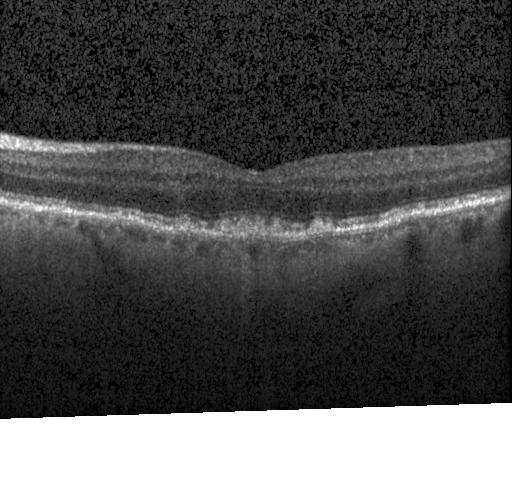

Macular OCT: multiple drusen.